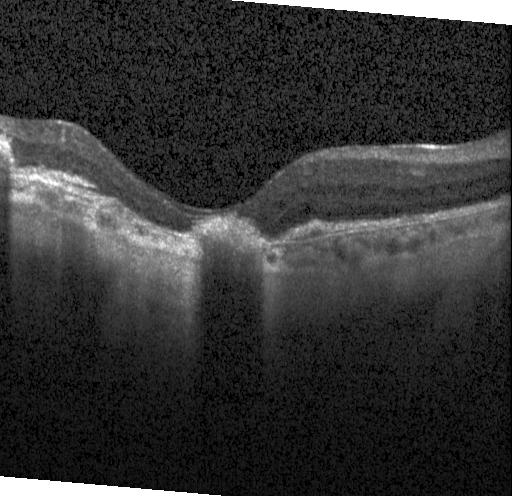

SD-OCT. Acquired on a Heidelberg Spectralis. OCT line scan — OCT finding: a choroidal neovascular membrane.